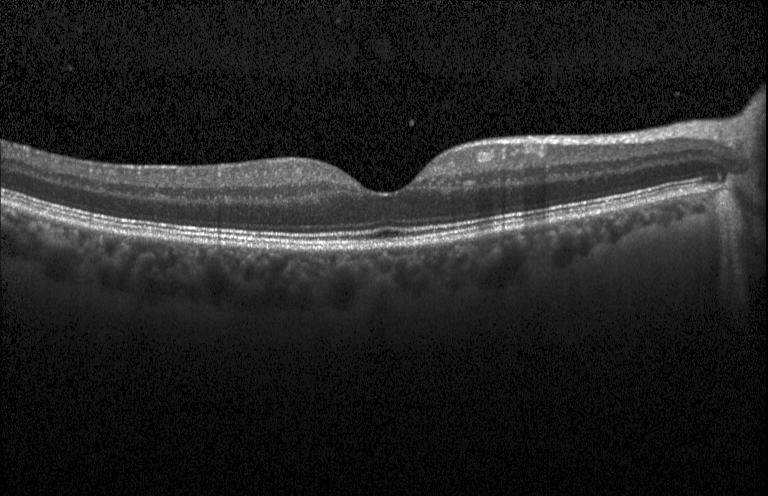 OCT B-scan showing neither CNV, DME, nor drusen.